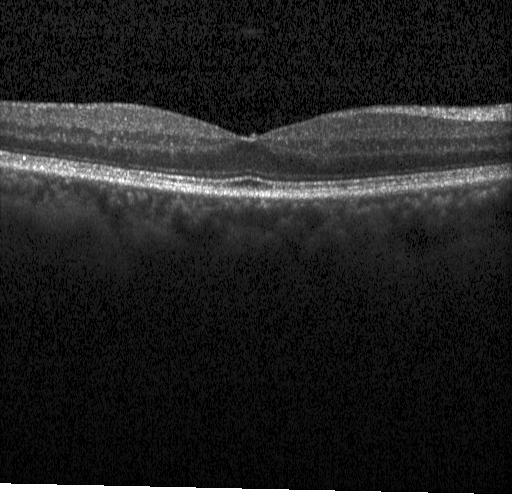
Retinal OCT cross-section
Macular OCT: no choroidal neovascularization, diabetic macular edema, or drusen.